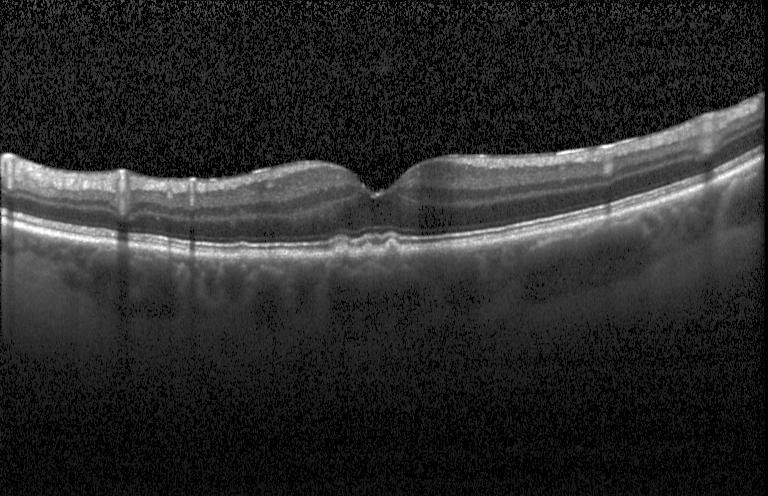

OCT B-scan showing drusen.